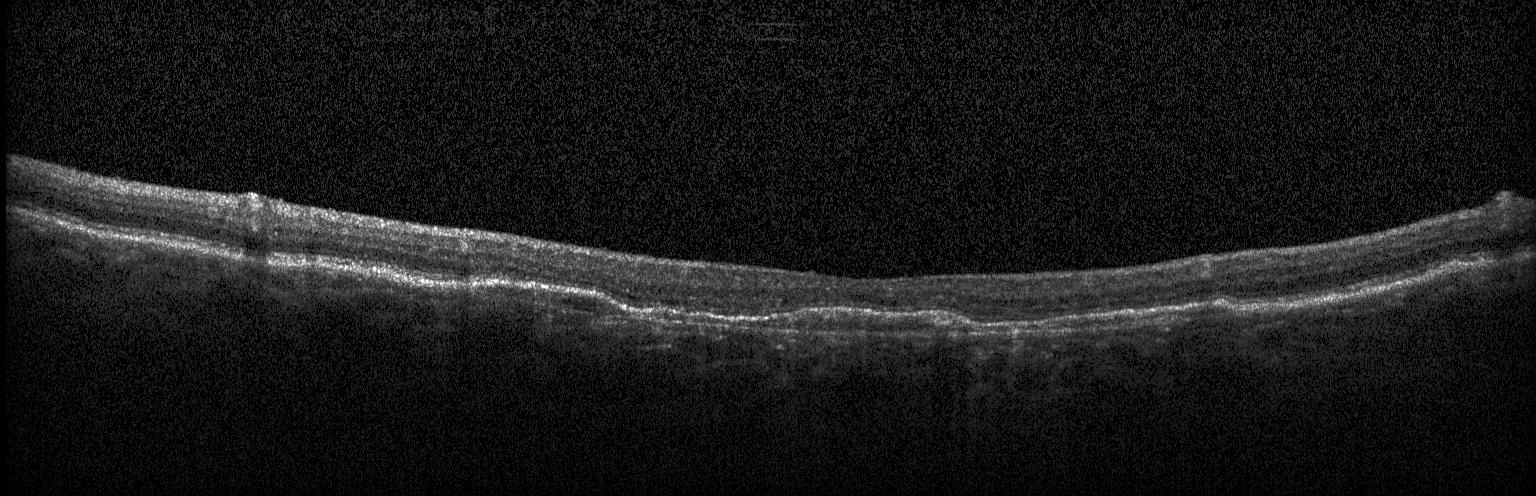
Spectral-domain OCT, optical coherence tomography B-scan, macular scan — Diagnosis: a choroidal neovascular membrane.